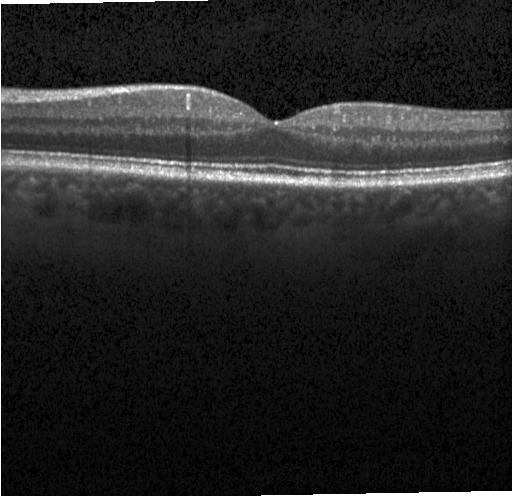

OCT line scan. The scan shows no evidence of choroidal neovascularization, diabetic macular edema, or drusen.